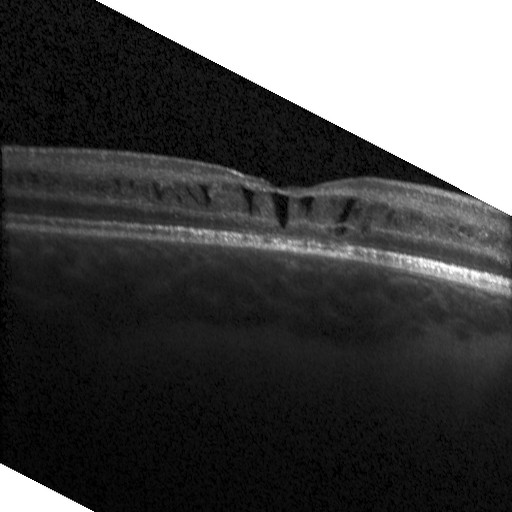 Heidelberg Spectralis OCT system, horizontal scan through the fovea, OCT line scan — Assessment: diabetic macular edema.